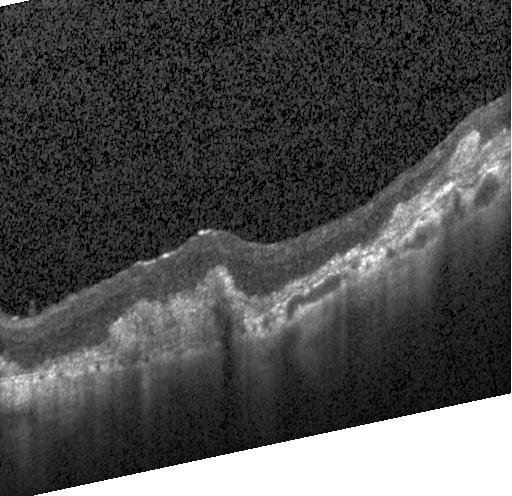 OCT line scan
Diagnosis: choroidal neovascularization (CNV).